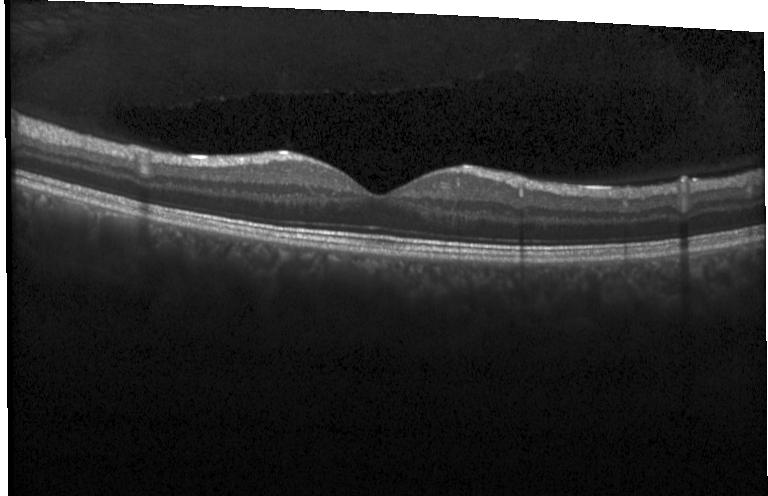

Macular OCT: no choroidal neovascularization, diabetic macular edema, or drusen.